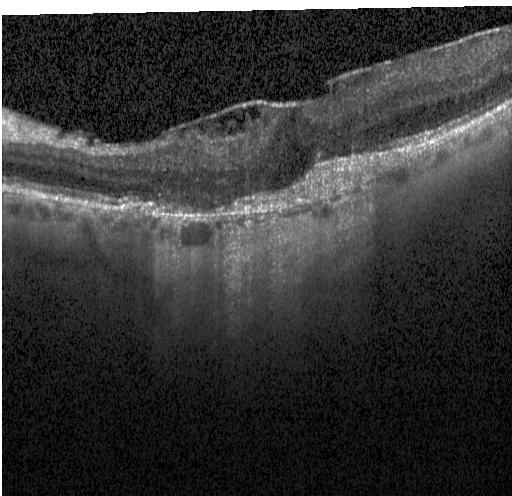

Optical coherence tomography B-scan. OCT finding: a choroidal neovascular membrane.